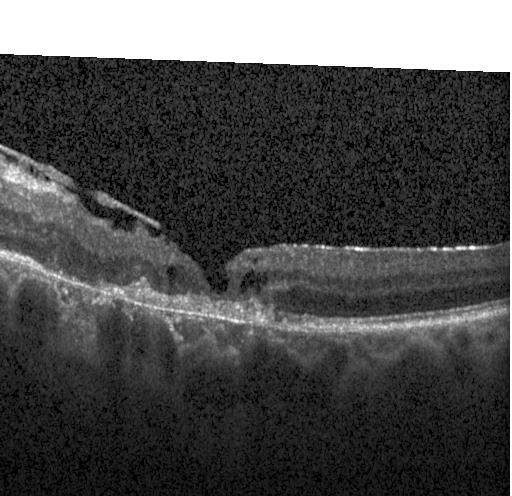

SD-OCT; optical coherence tomography B-scan.
Finding: CNV.